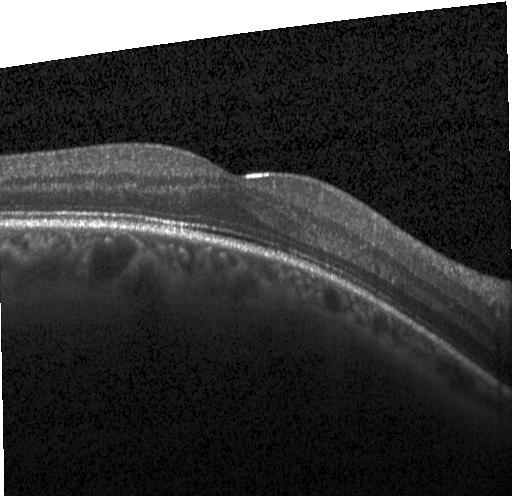 Optical coherence tomography B-scan
Finding: neither choroidal neovascularization, diabetic macular edema, nor drusen.